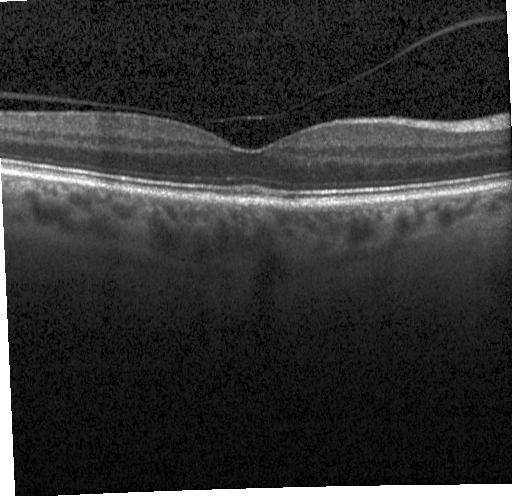

Optical coherence tomography B-scan, macular scan — Finding: no evidence of choroidal neovascularization, diabetic macular edema, or drusen.